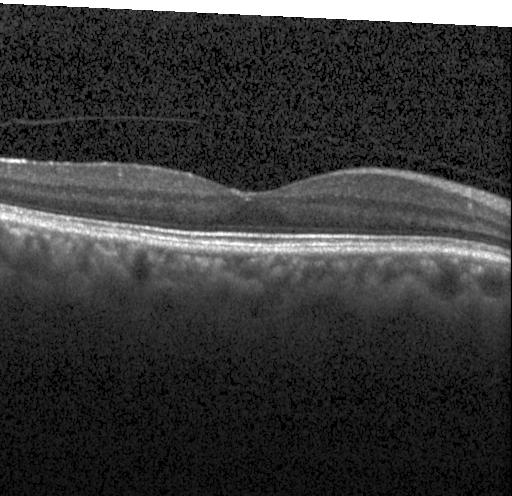
Retinal OCT cross-section. Impression: no choroidal neovascularization, no diabetic macular edema, and no drusen.